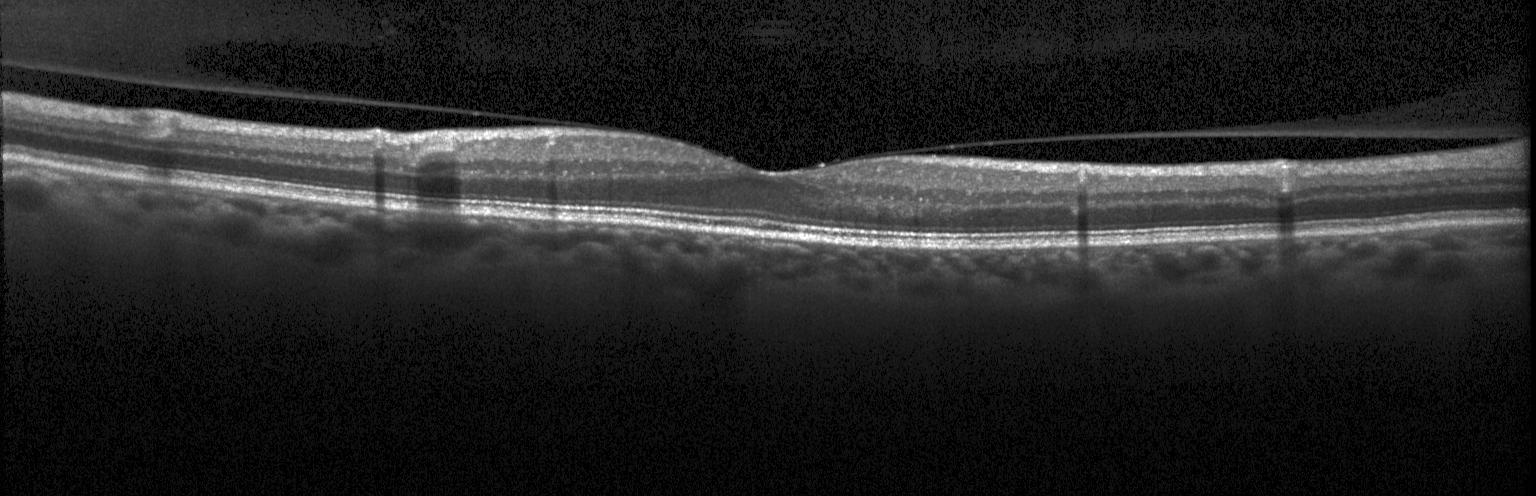 Macular OCT demonstrating no choroidal neovascularization, diabetic macular edema, or drusen.